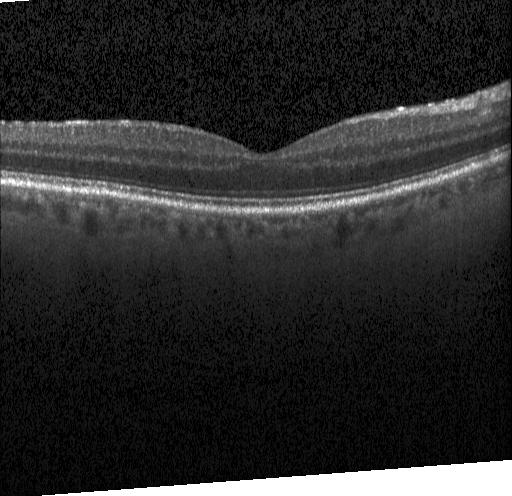 Acquired on a Heidelberg Spectralis. Optical coherence tomography B-scan. Fovea-centered
Macular OCT: no CNV, DME, or drusen.